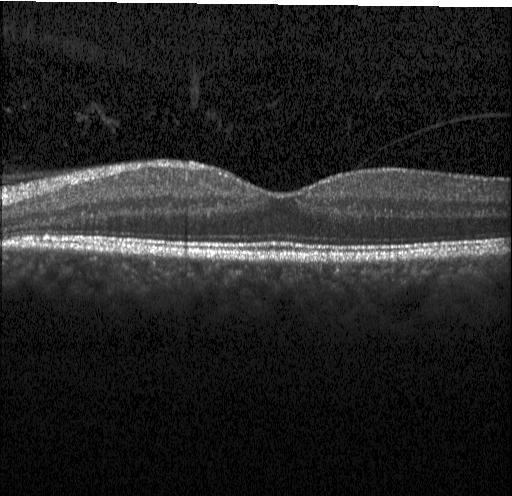
Impression: neither choroidal neovascularization, diabetic macular edema, nor drusen.